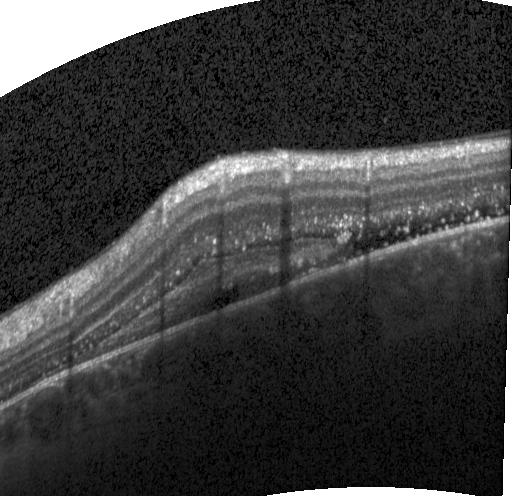

Retinal OCT B-scan · instrument: Heidelberg Spectralis · horizontal scan through the fovea. Assessment: choroidal neovascularization (CNV).